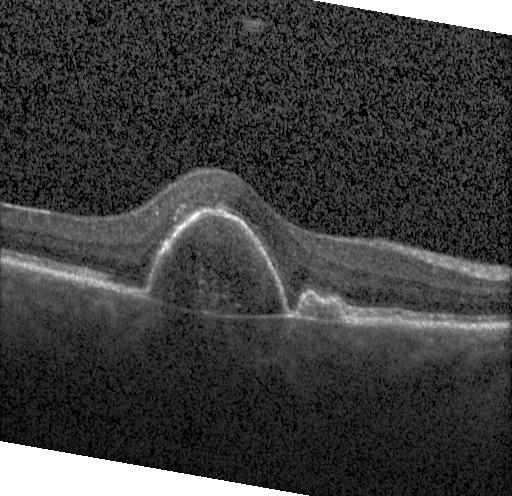

OCT B-scan; SD-OCT — Finding: a choroidal neovascular membrane.